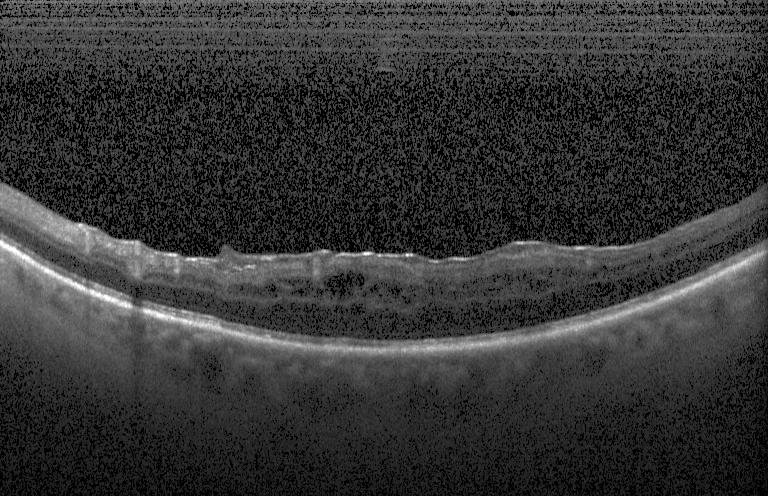
OCT B-scan — Finding: diabetic macular edema (DME).